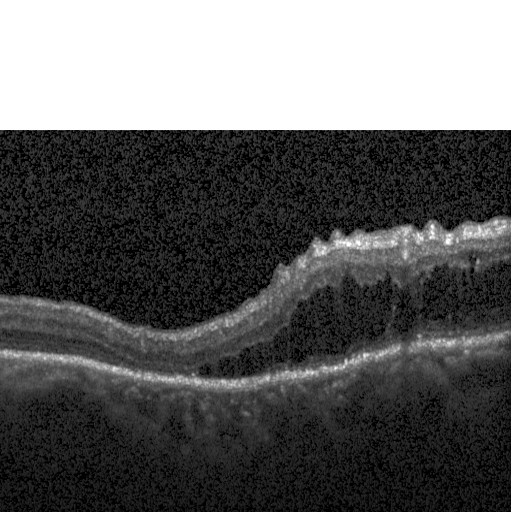

Optical coherence tomography B-scan — Dx: diabetic macular edema.